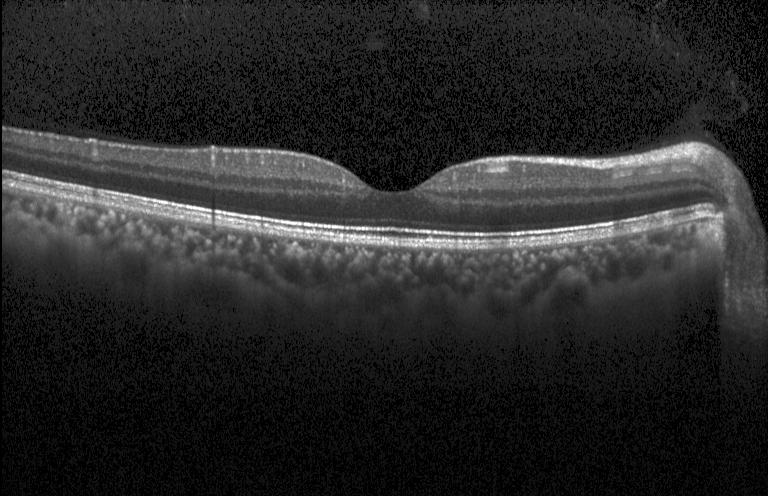 Finding: neither choroidal neovascularization, diabetic macular edema, nor drusen.